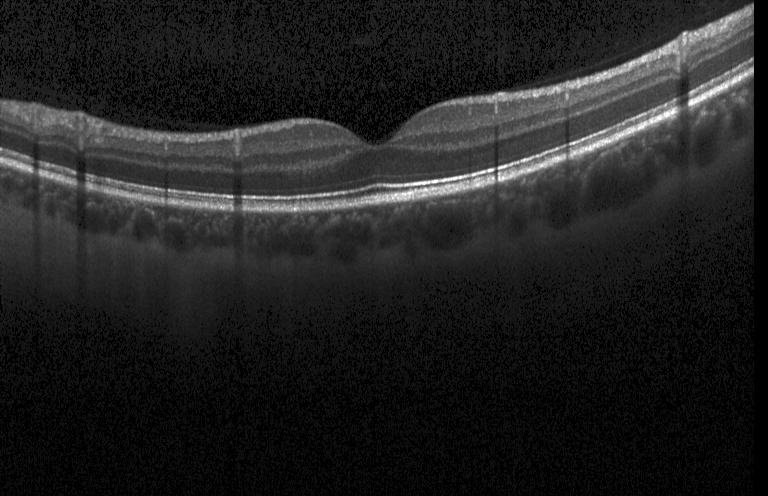 Diagnosis: neither CNV, DME, nor drusen.